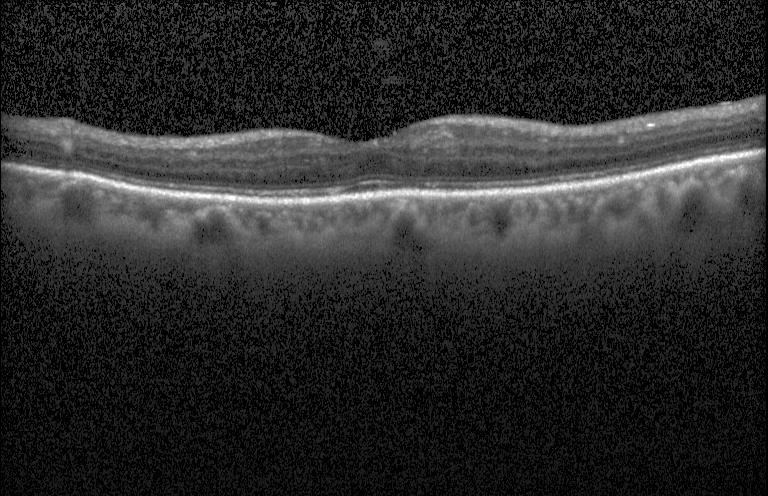

Impression: no evidence of choroidal neovascularization, diabetic macular edema, or drusen.